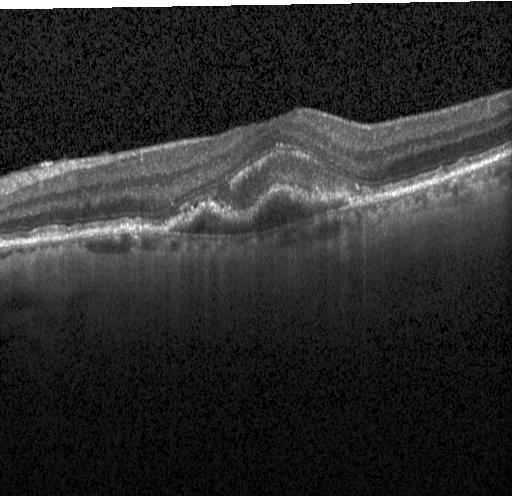

OCT finding: a choroidal neovascular membrane.